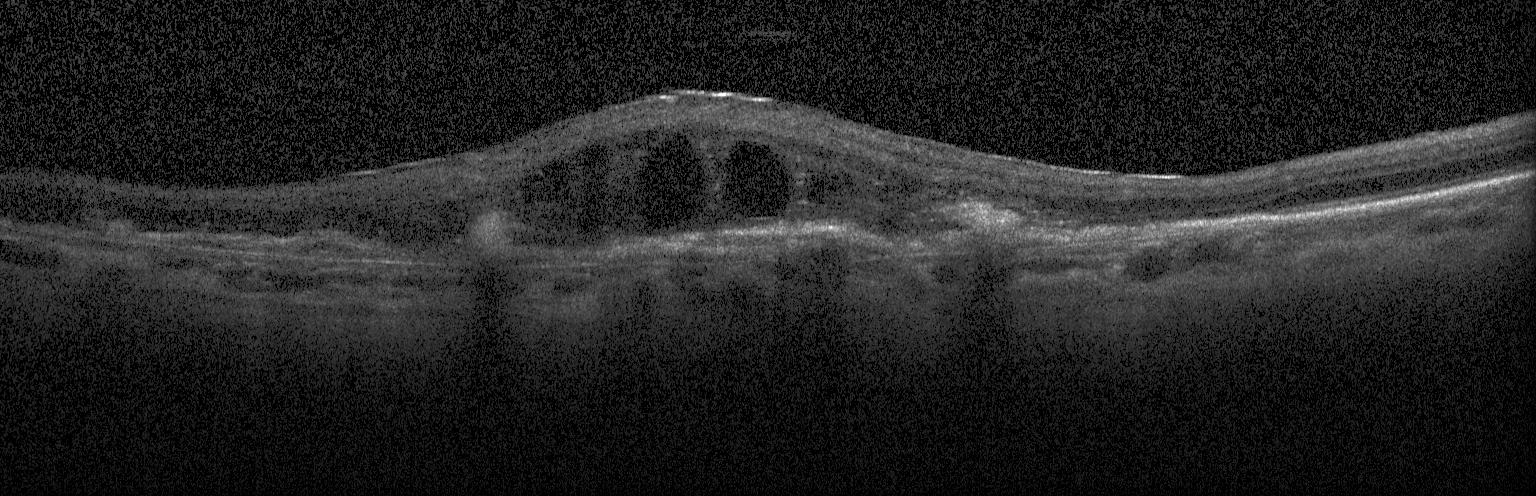
The scan shows choroidal neovascularization.